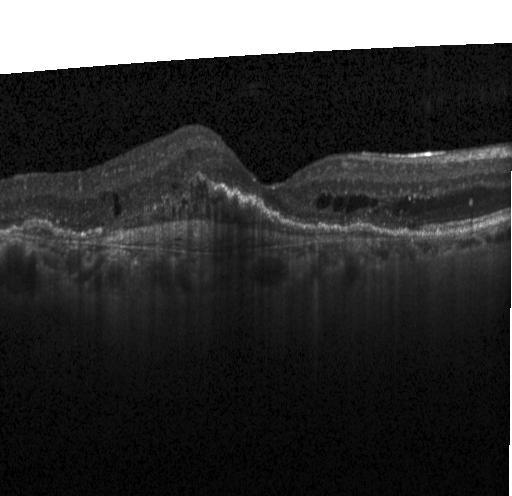
The scan shows CNV.